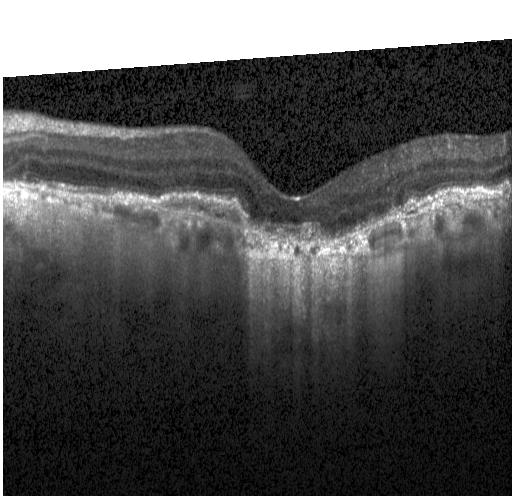
Retinal OCT B-scan — Finding: CNV.